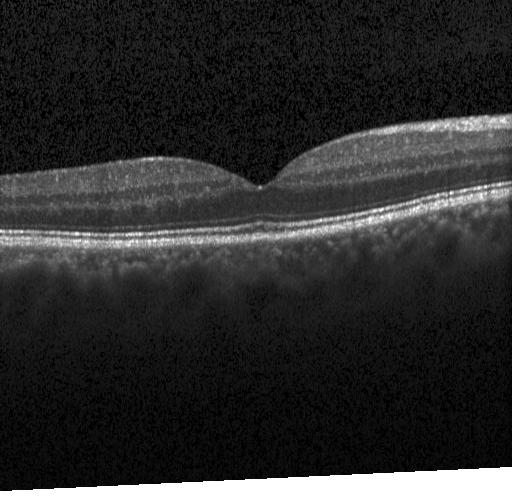
Optical coherence tomography B-scan · fovea-centered · Heidelberg Spectralis.
The scan shows neither CNV, DME, nor drusen.